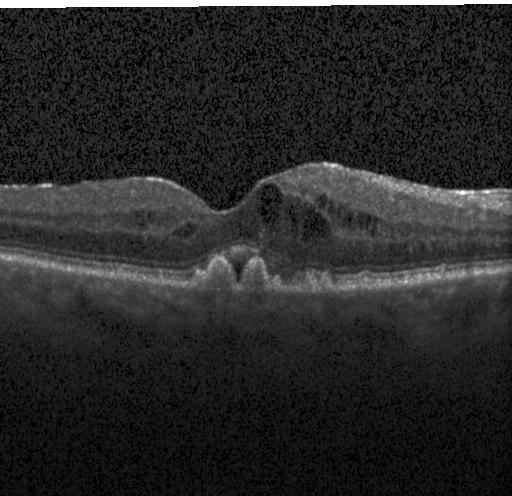 OCT B-scan. Assessment: a choroidal neovascular membrane.